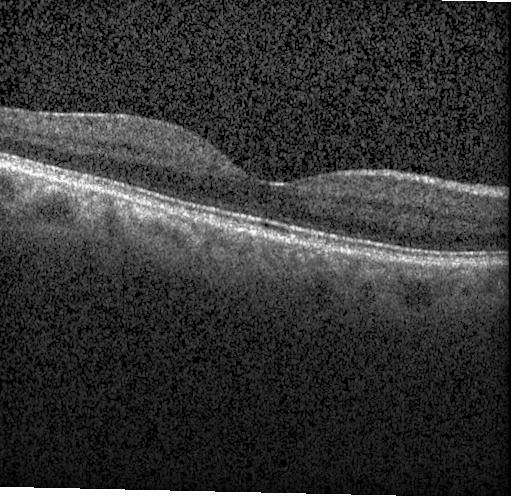
Horizontal scan through the fovea, Heidelberg Spectralis, SD-OCT, retinal OCT B-scan
Impression: neither choroidal neovascularization, diabetic macular edema, nor drusen.